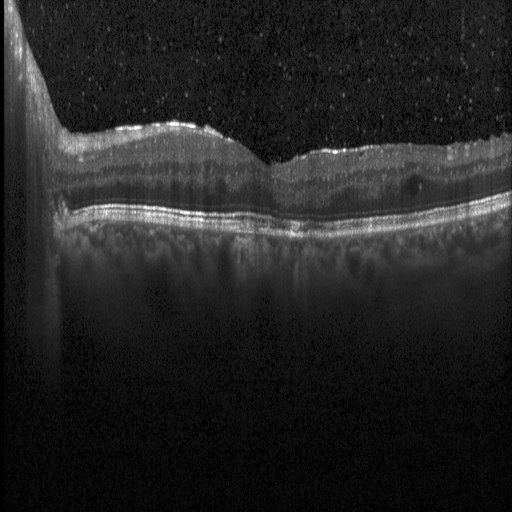
Fovea-centered, retinal OCT B-scan, Heidelberg Spectralis OCT system, spectral-domain optical coherence tomography
This B-scan demonstrates diabetic macular edema (DME).